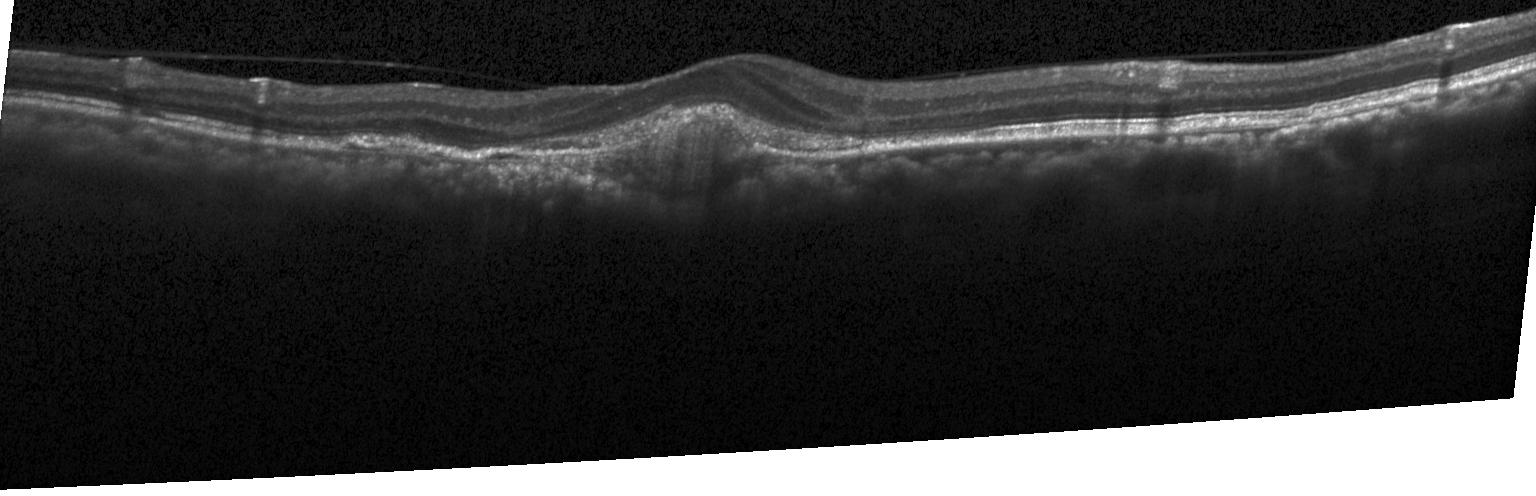
Instrument: Heidelberg Spectralis; horizontal scan through the fovea; spectral-domain optical coherence tomography; retinal OCT cross-section. This B-scan demonstrates a choroidal neovascular membrane.